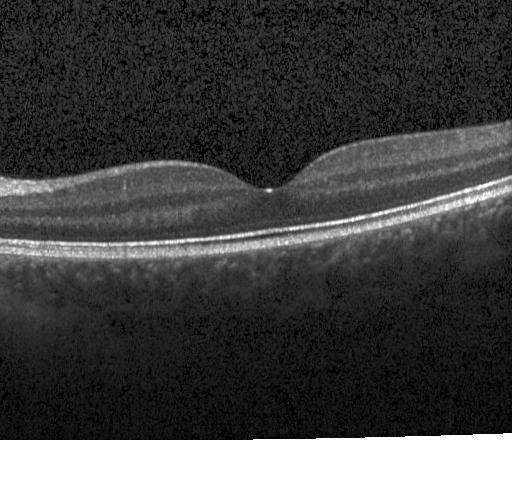
SD-OCT, retinal OCT cross-section — This B-scan demonstrates no evidence of choroidal neovascularization, diabetic macular edema, or drusen.